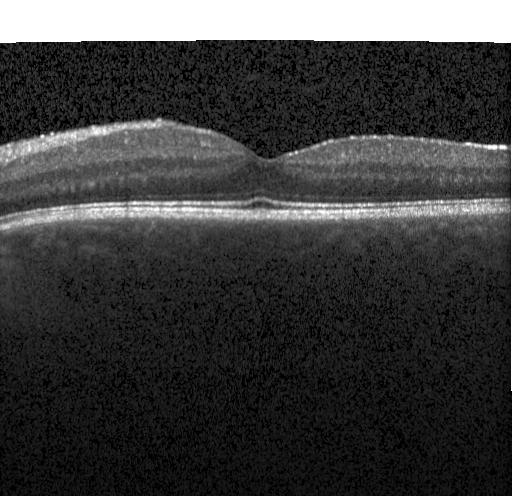
OCT B-scan.
Macular OCT: no choroidal neovascularization, diabetic macular edema, or drusen.